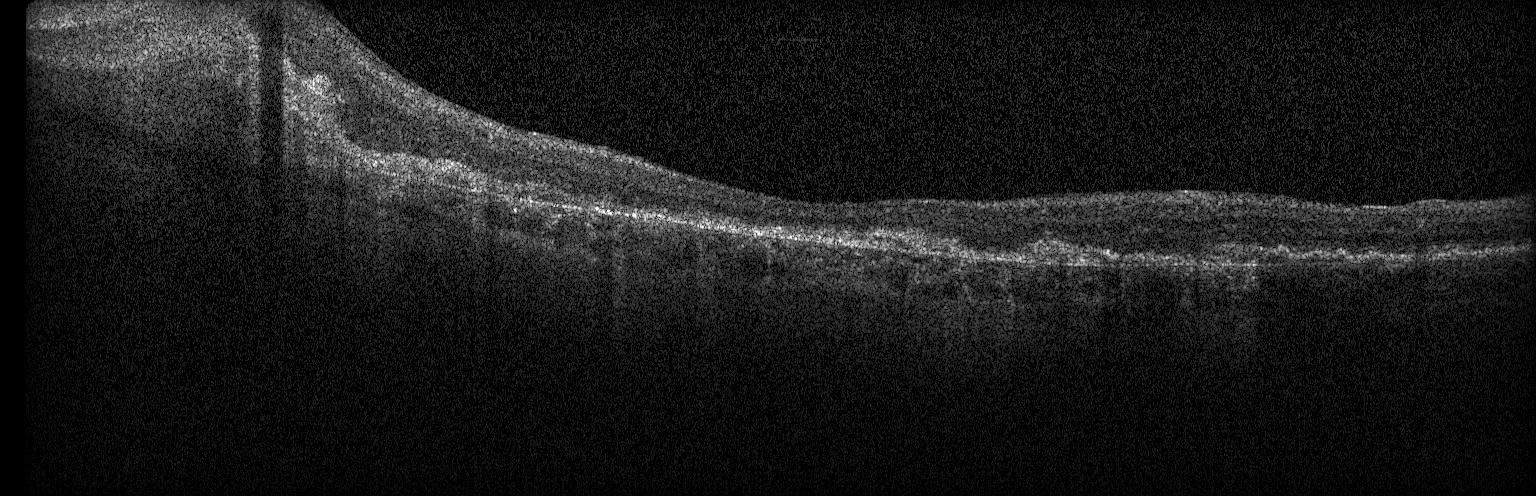
Spectral-domain OCT; centered on the fovea; optical coherence tomography scan; instrument: Heidelberg Spectralis
Diagnosis: a choroidal neovascular membrane.